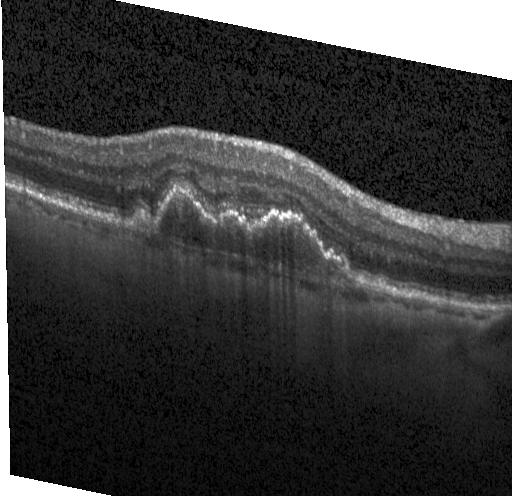 Heidelberg Spectralis OCT system · fovea-centered · spectral-domain optical coherence tomography · optical coherence tomography scan.
Macular OCT: choroidal neovascularization (CNV).